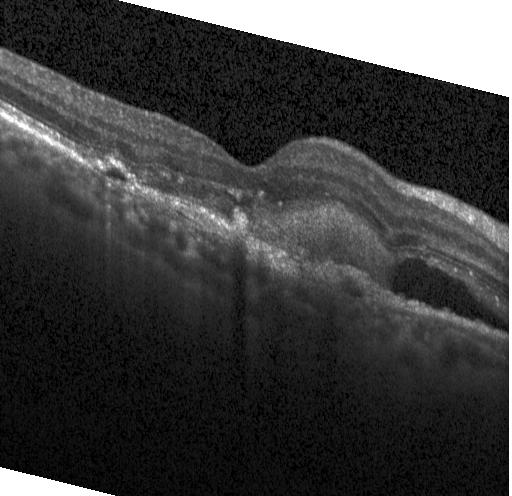

Retinal OCT cross-section
The scan shows CNV.